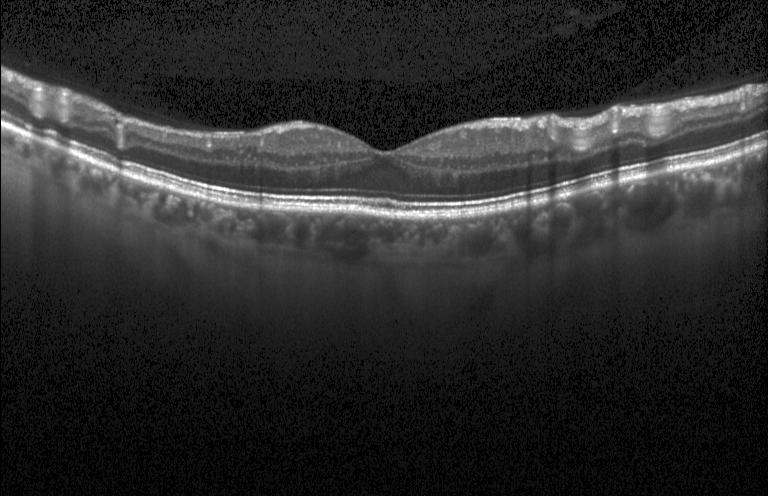 Retinal OCT B-scan
Impression: no evidence of choroidal neovascularization, diabetic macular edema, or drusen.